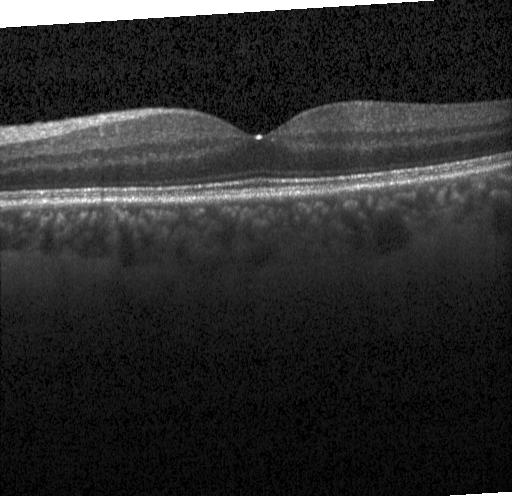
Retinal OCT cross-section
Impression: neither choroidal neovascularization, diabetic macular edema, nor drusen.